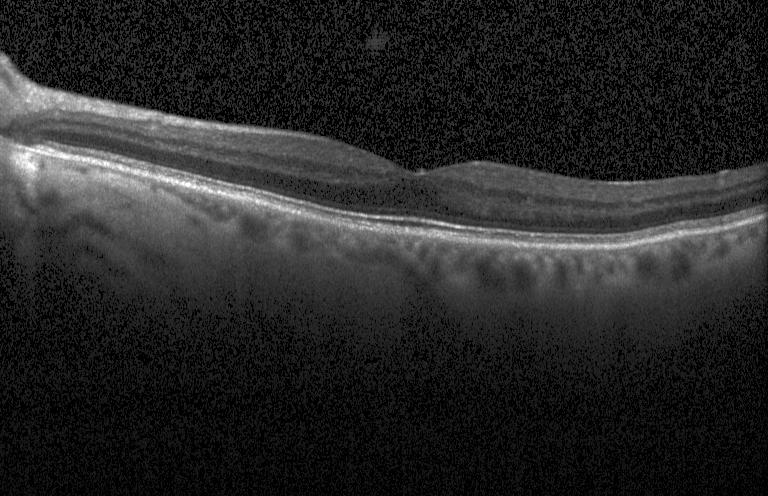 Spectral-domain OCT B-scan: neither choroidal neovascularization, diabetic macular edema, nor drusen.